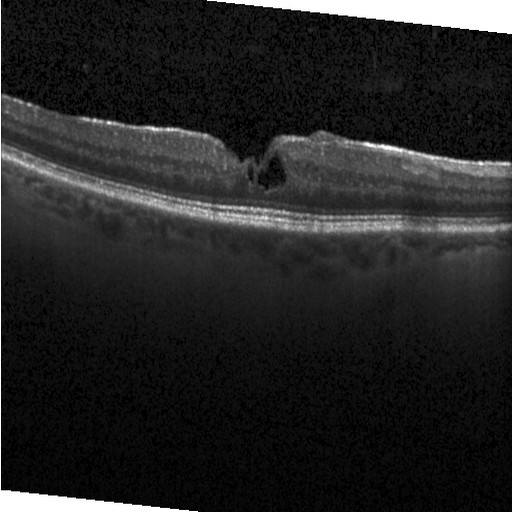
Retinal OCT cross-section showing DME.